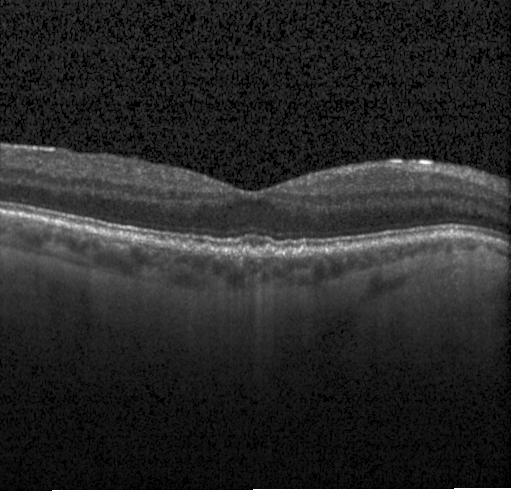 Macular scan. Instrument: Heidelberg Spectralis. Optical coherence tomography B-scan. SD-OCT — Impression: sub-RPE drusenoid deposits.